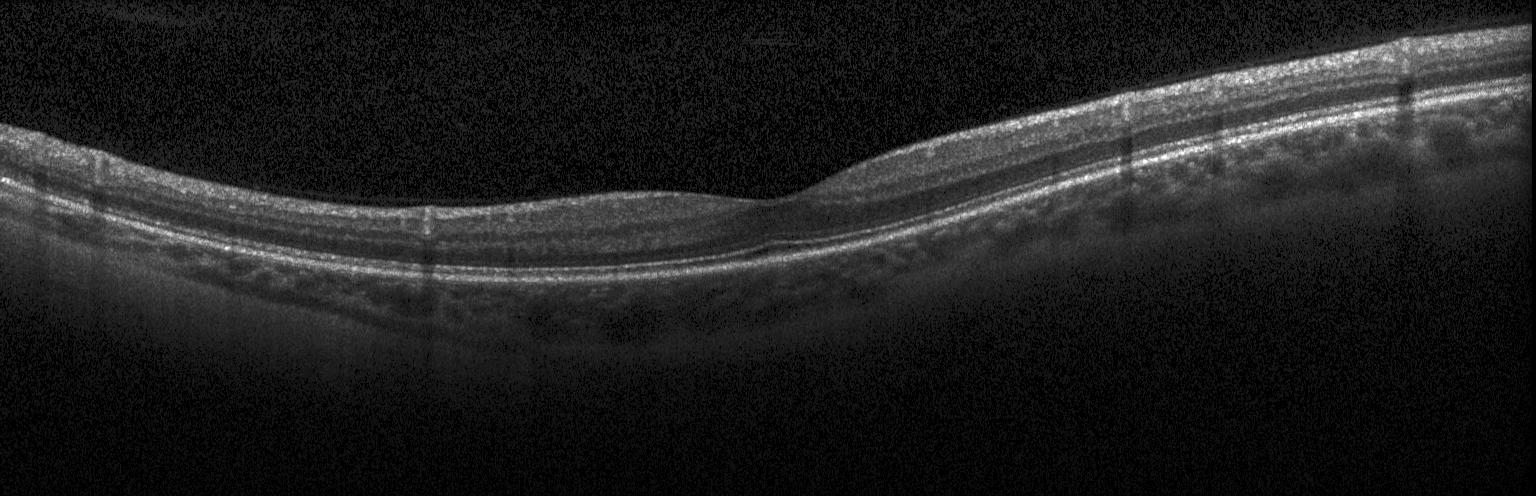

Through the macula; spectral-domain OCT; retinal OCT B-scan.
The scan shows no CNV, no DME, and no drusen.